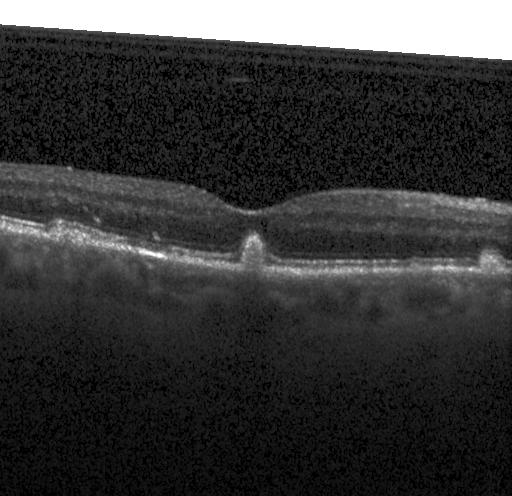
Retinal OCT cross-section, spectral-domain OCT — Diagnosis: sub-RPE drusenoid deposits.